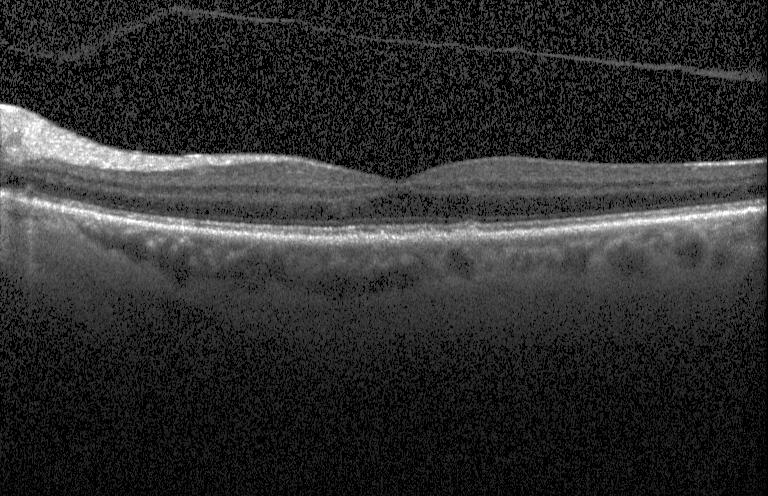 Impression: sub-RPE drusenoid deposits.